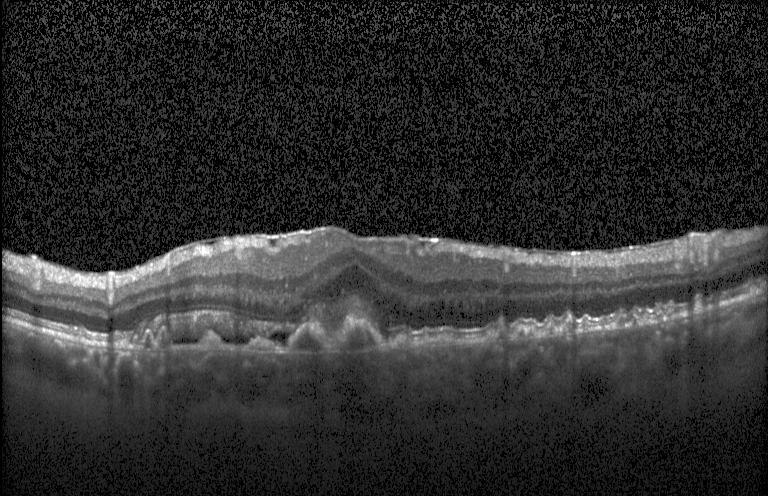 Finding: choroidal neovascularization.